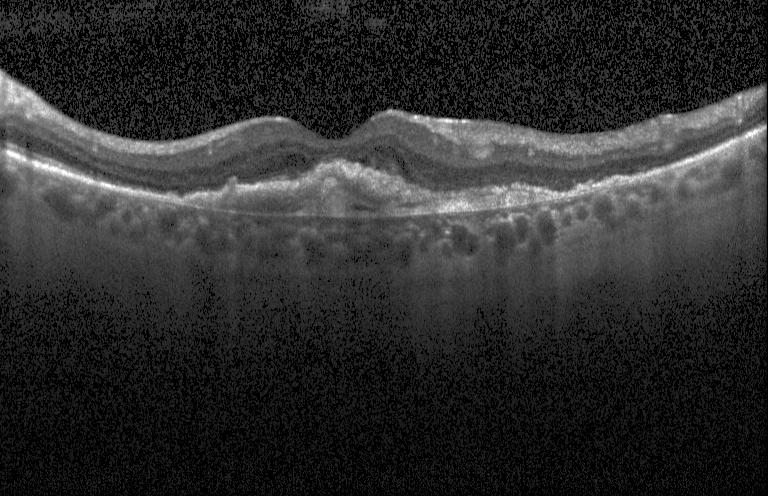

Dx: a choroidal neovascular membrane.